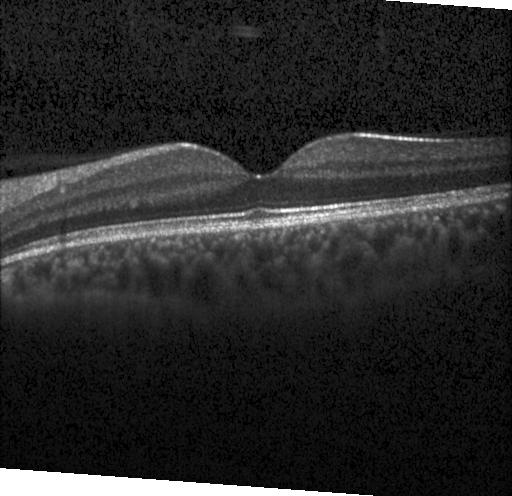 Retinal OCT cross-section · spectral-domain OCT. Impression: neither choroidal neovascularization, diabetic macular edema, nor drusen.